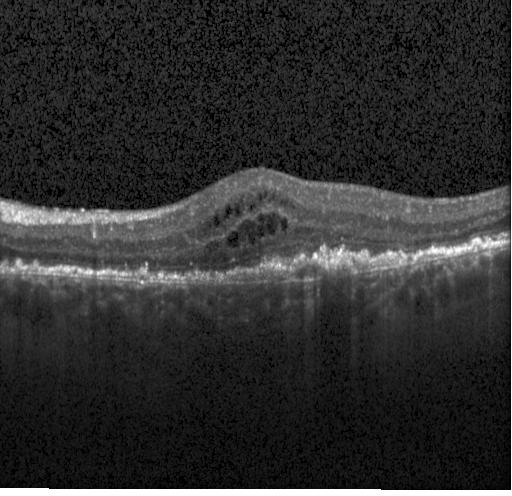 Diagnosis: choroidal neovascularization (CNV).